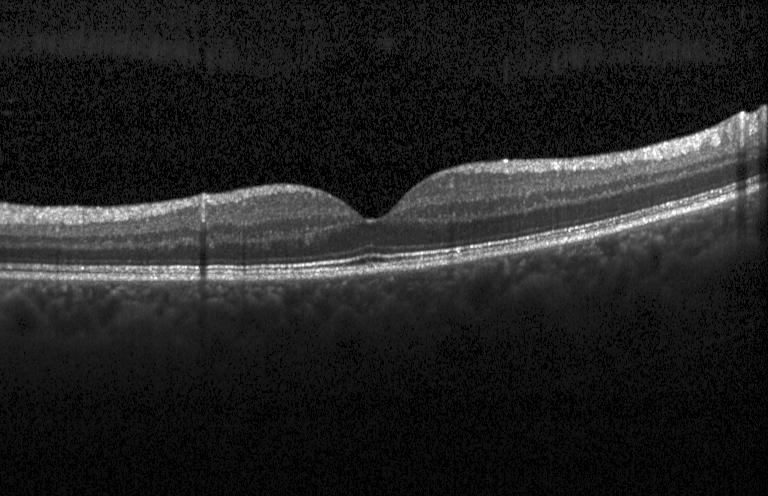
Spectral-domain OCT · centered on the fovea · OCT B-scan · Heidelberg Spectralis OCT system
Impression: no choroidal neovascularization, diabetic macular edema, or drusen.